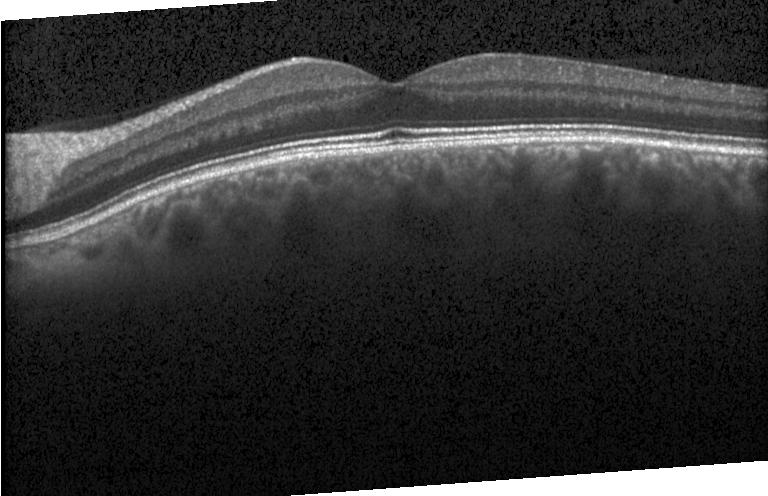

Diagnosis: no choroidal neovascularization, no diabetic macular edema, and no drusen.